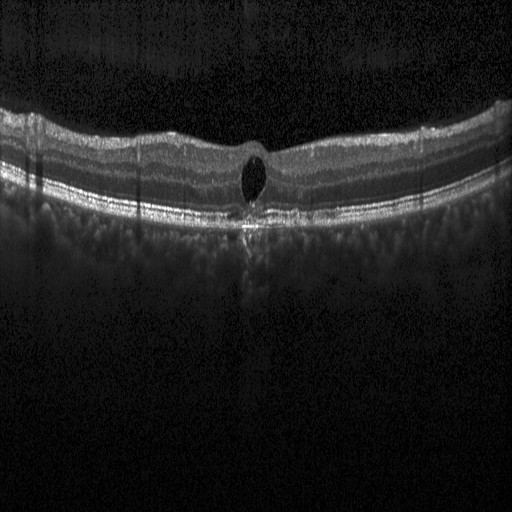
Instrument: Heidelberg Spectralis, retinal OCT B-scan, SD-OCT, through the macula.
Finding: DME.